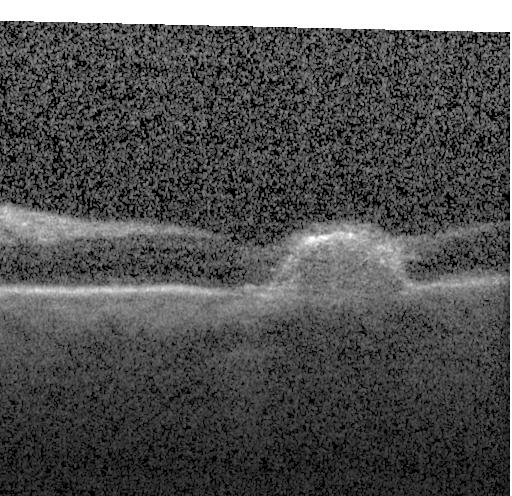 Macular OCT: choroidal neovascularization (CNV).